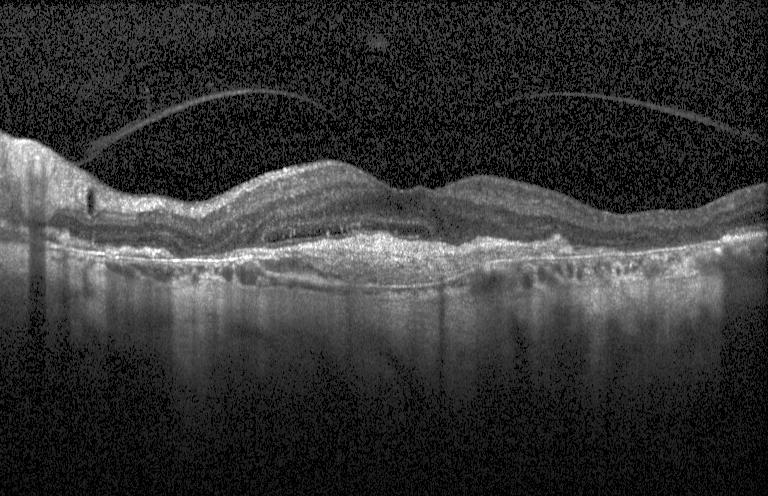

OCT B-scan showing a choroidal neovascular membrane.